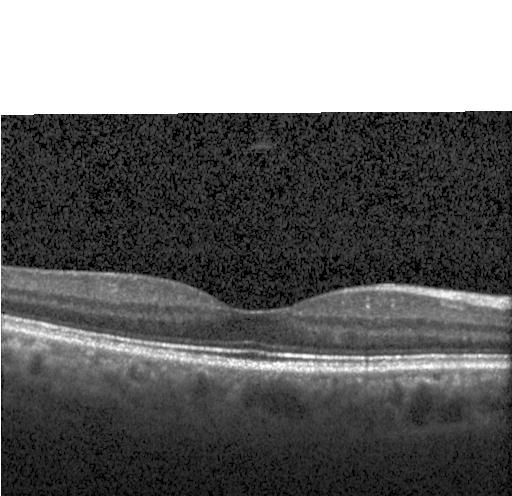

Through the macula. Optical coherence tomography scan. Finding: no choroidal neovascularization, diabetic macular edema, or drusen.